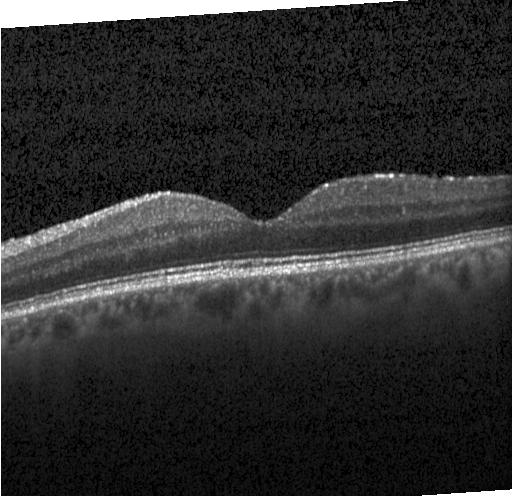

Acquired on a Heidelberg Spectralis, optical coherence tomography B-scan — This B-scan demonstrates no choroidal neovascularization, diabetic macular edema, or drusen.